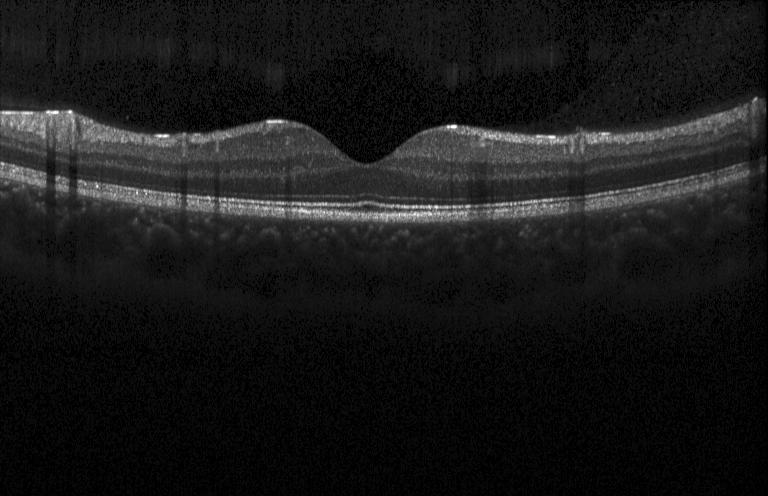 OCT scan showing no evidence of choroidal neovascularization, diabetic macular edema, or drusen.